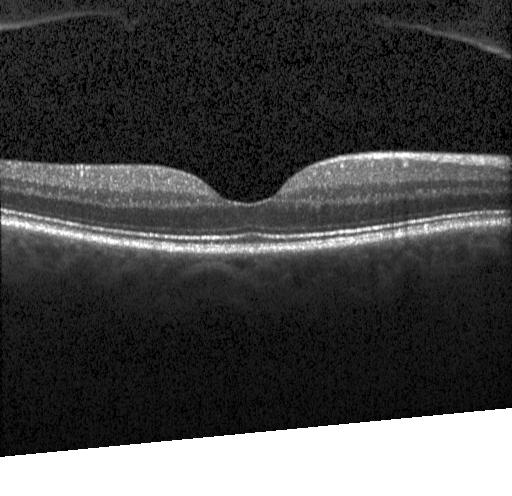

Neither choroidal neovascularization, diabetic macular edema, nor drusen.